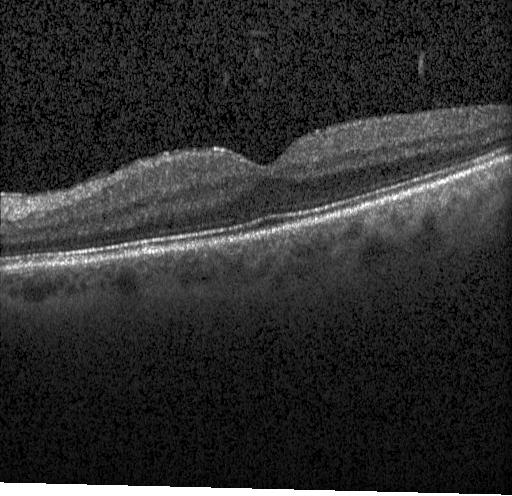 Optical coherence tomography B-scan. Macular scan. The scan shows no CNV, DME, or drusen.